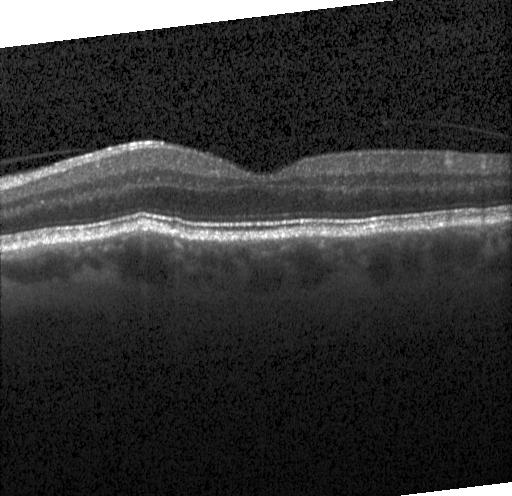

Macular OCT: no choroidal neovascularization, no diabetic macular edema, and no drusen.